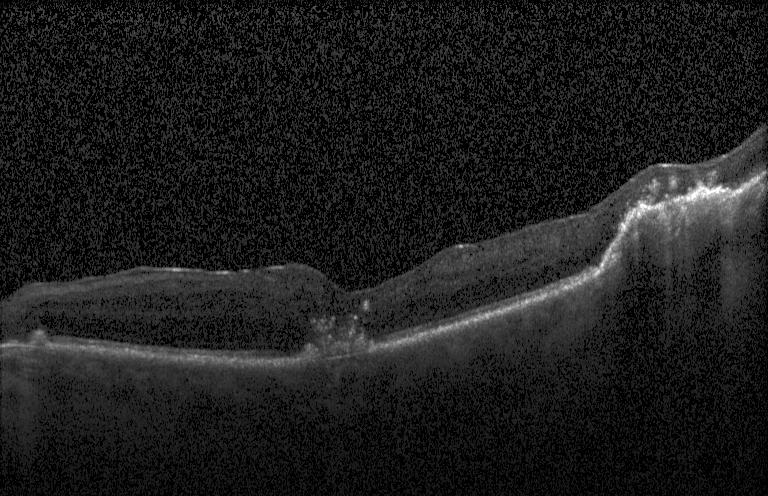
Spectral-domain optical coherence tomography · OCT B-scan · acquired on a Heidelberg Spectralis — Choroidal neovascularization (CNV).